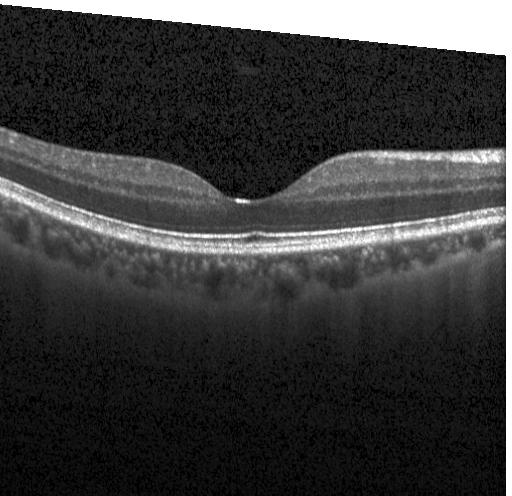
SD-OCT, OCT B-scan, centered on the fovea, acquired on a Heidelberg Spectralis.
Finding: no choroidal neovascularization, diabetic macular edema, or drusen.